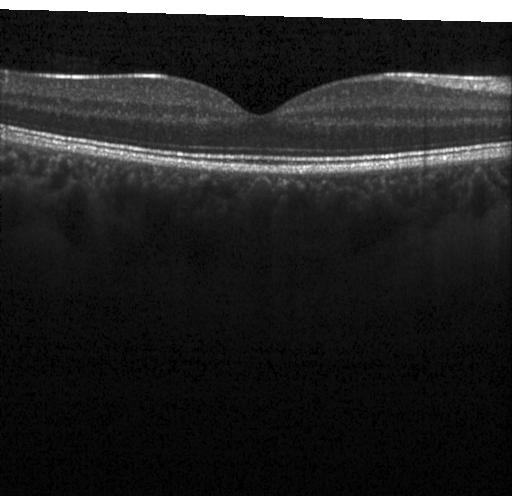

Heidelberg Spectralis OCT system. Optical coherence tomography scan — Impression: no choroidal neovascularization, no diabetic macular edema, and no drusen.